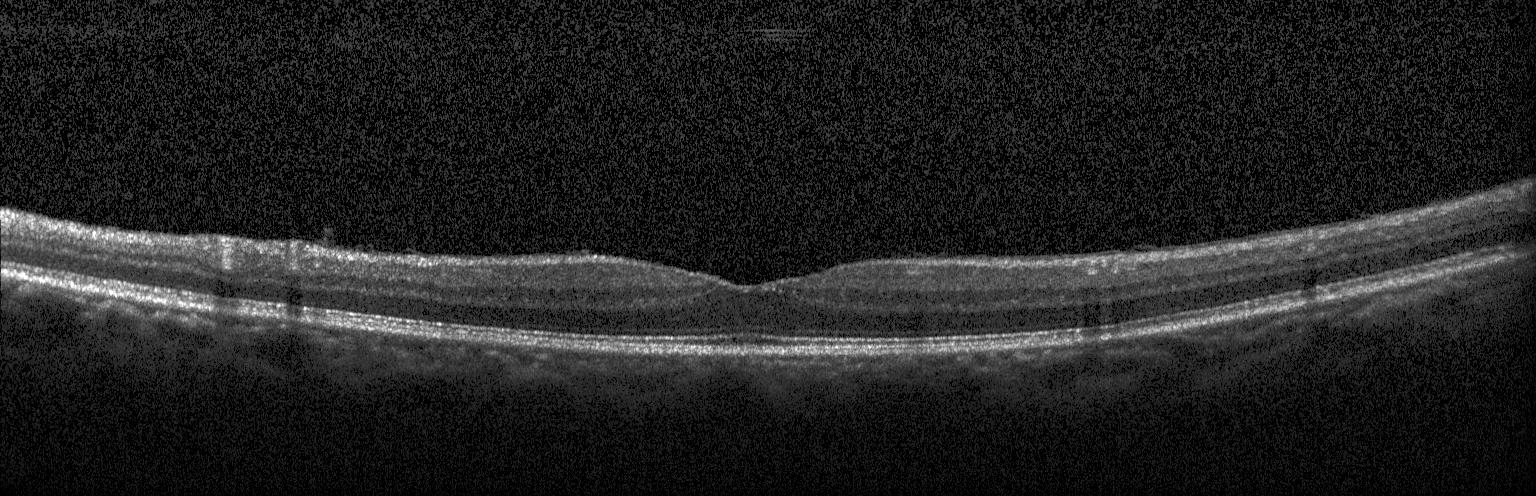

Retinal OCT cross-section
No choroidal neovascularization, diabetic macular edema, or drusen.